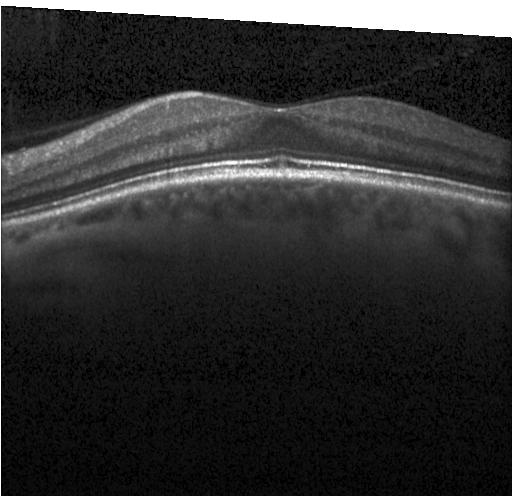

OCT finding: no choroidal neovascularization, diabetic macular edema, or drusen.